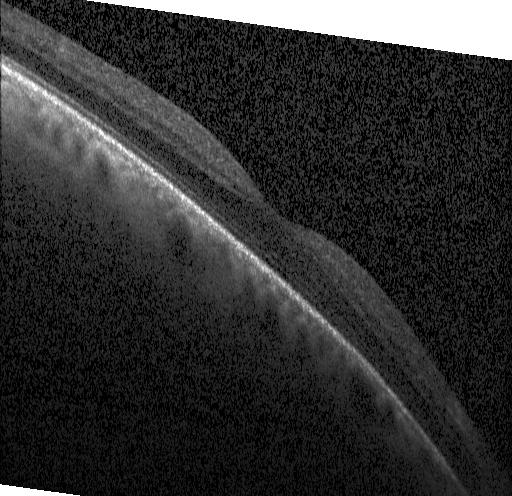

Assessment: no evidence of choroidal neovascularization, diabetic macular edema, or drusen.